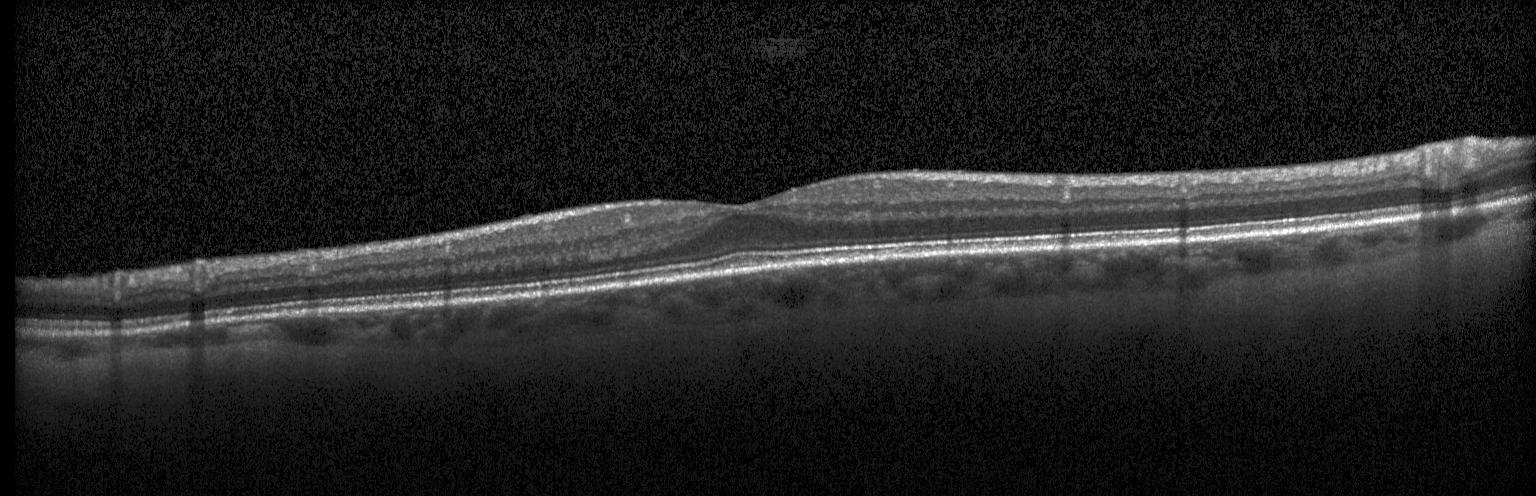

SD-OCT · horizontal scan through the fovea · acquired on a Heidelberg Spectralis · retinal OCT B-scan — Finding: no choroidal neovascularization, diabetic macular edema, or drusen.